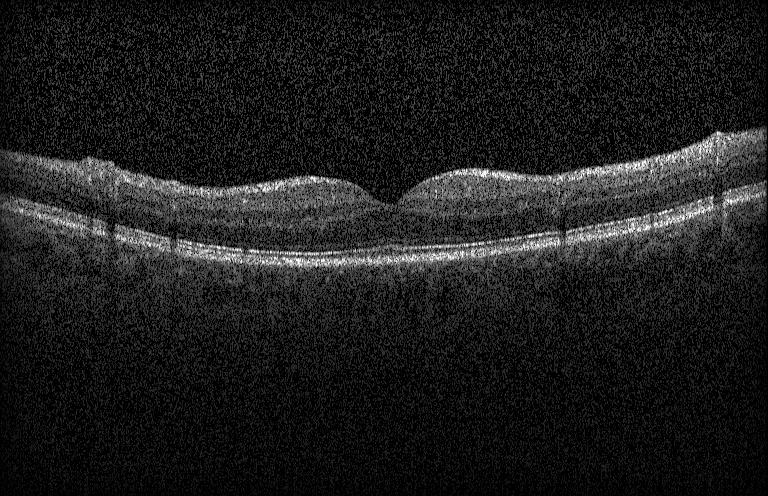 Macular OCT: neither CNV, DME, nor drusen.